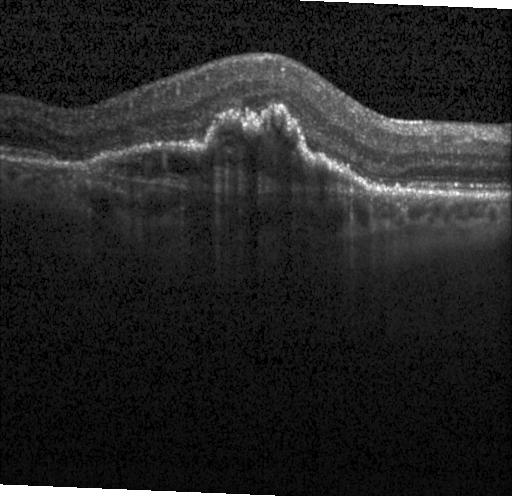

SD-OCT · optical coherence tomography scan — Finding: a choroidal neovascular membrane.